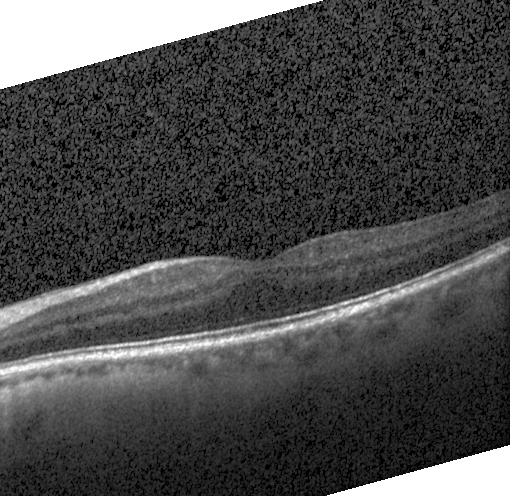

Finding: no choroidal neovascularization, no diabetic macular edema, and no drusen.